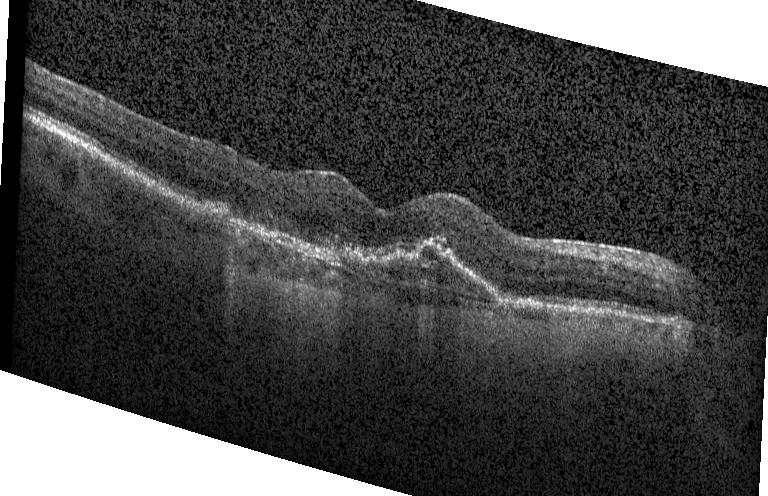
OCT finding: CNV.